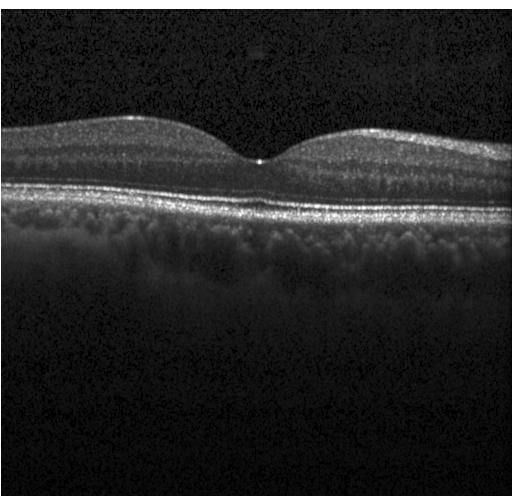

Macular OCT: neither choroidal neovascularization, diabetic macular edema, nor drusen.